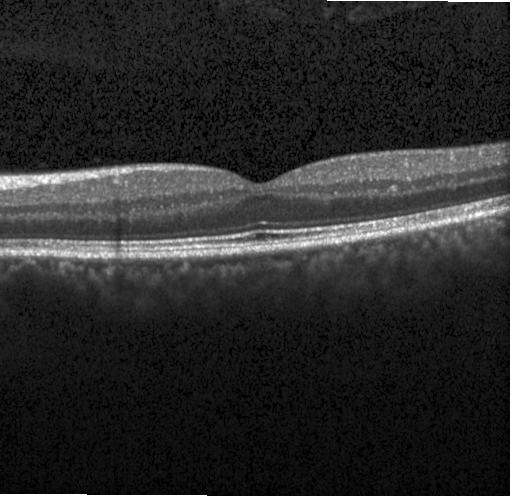

Retinal OCT cross-section showing neither choroidal neovascularization, diabetic macular edema, nor drusen.